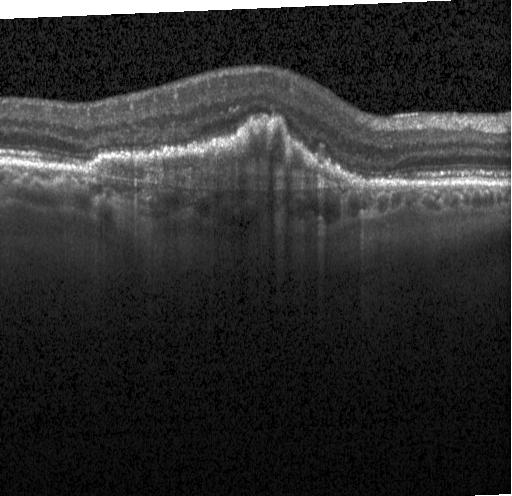 Finding: a choroidal neovascular membrane.